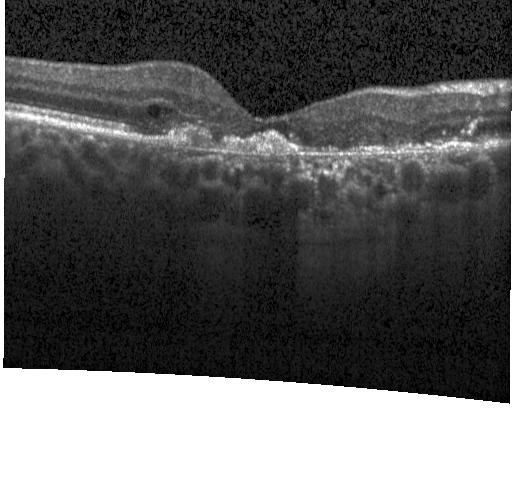 Dx: a choroidal neovascular membrane.